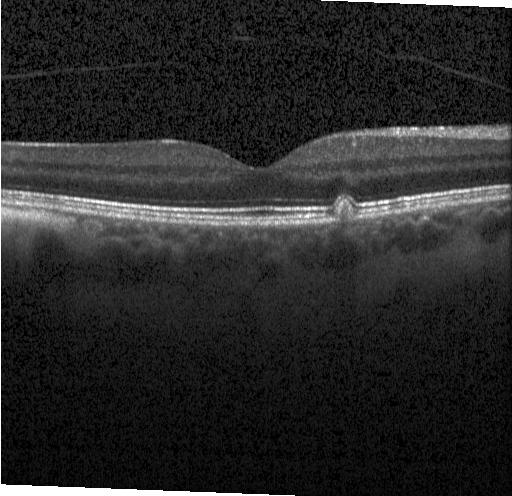 Retinal OCT B-scan; spectral-domain optical coherence tomography. Diagnosis: drusen.